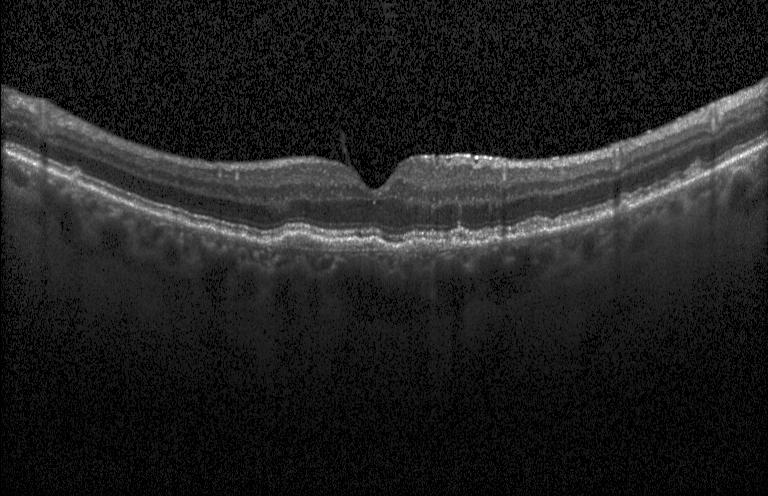

The scan shows a choroidal neovascular membrane.